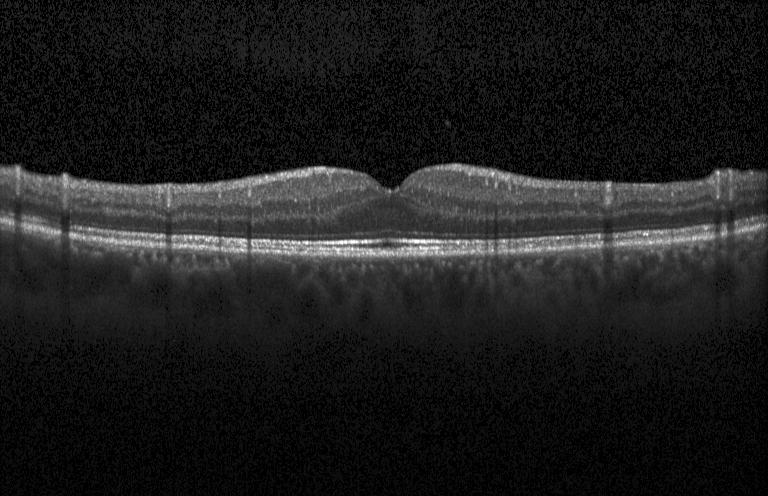

Optical coherence tomography scan · spectral-domain OCT · through the macula
Finding: neither choroidal neovascularization, diabetic macular edema, nor drusen.